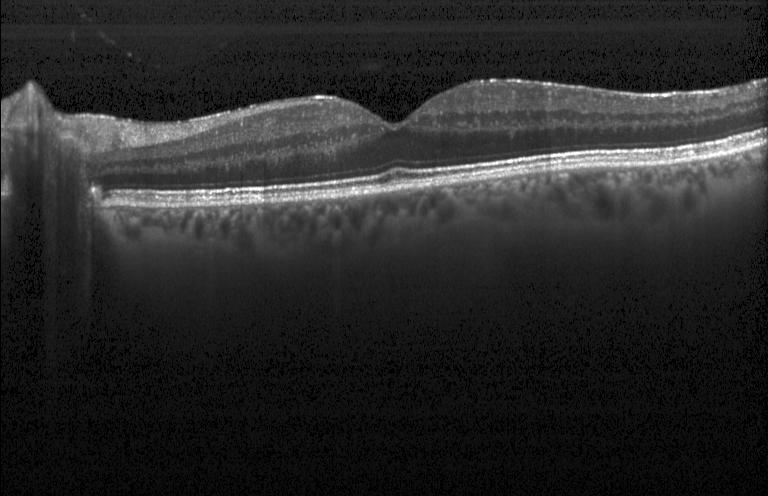

Macular scan; SD-OCT; OCT B-scan; Heidelberg Spectralis — The scan shows neither CNV, DME, nor drusen.